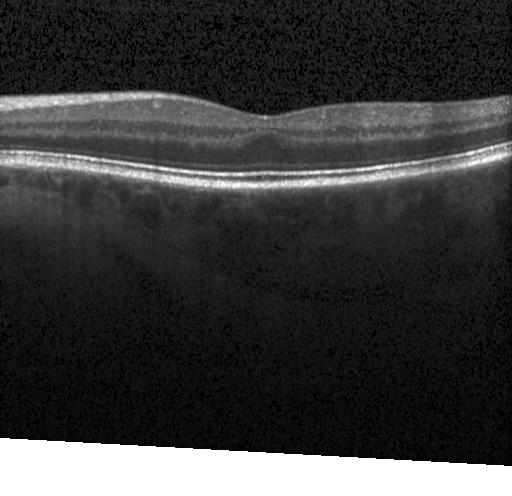
Heidelberg Spectralis; optical coherence tomography B-scan. Diagnosis: no choroidal neovascularization, diabetic macular edema, or drusen.